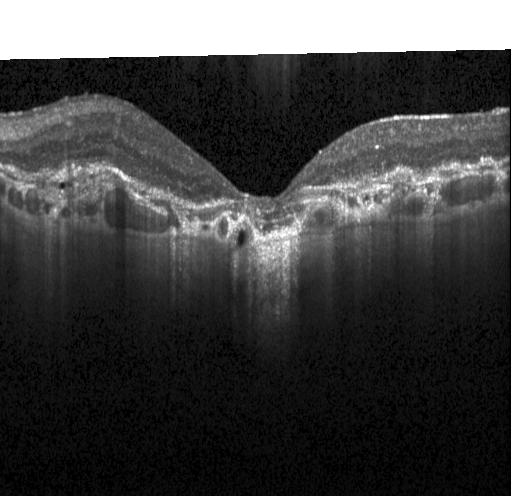 Diagnosis: a choroidal neovascular membrane.